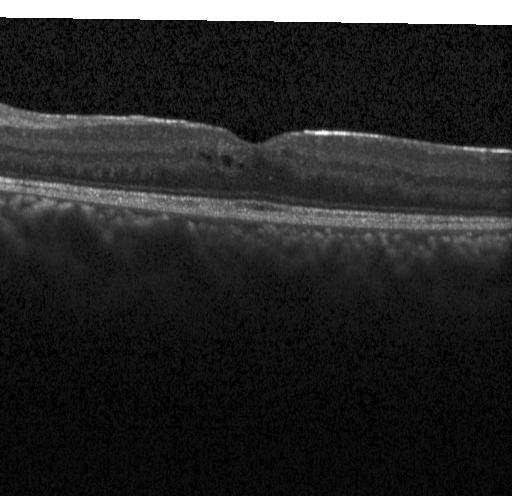

Optical coherence tomography scan — Impression: diabetic macular edema.